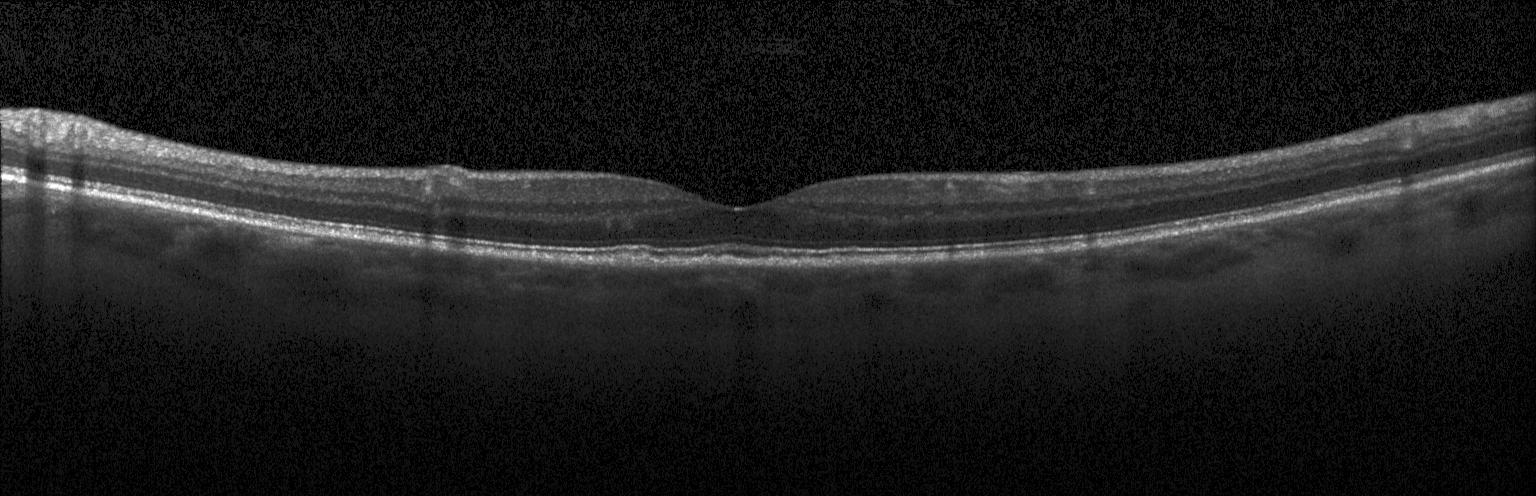

Acquired on a Heidelberg Spectralis, spectral-domain OCT, OCT line scan.
Dx: multiple drusen.